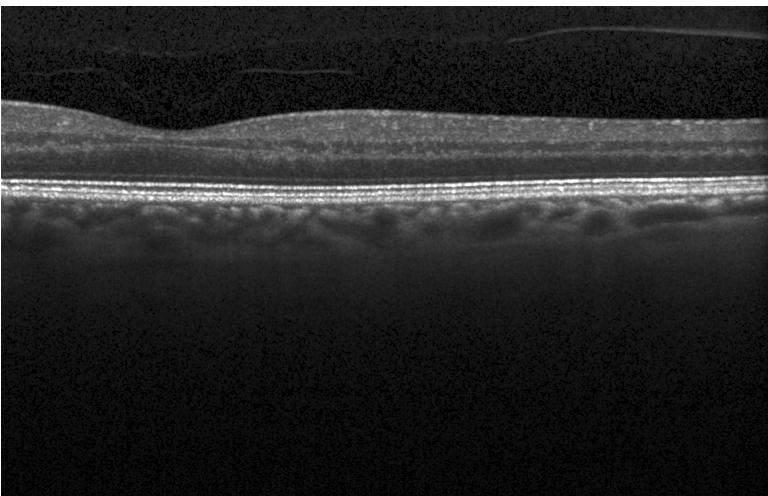 Dx: no evidence of choroidal neovascularization, diabetic macular edema, or drusen.